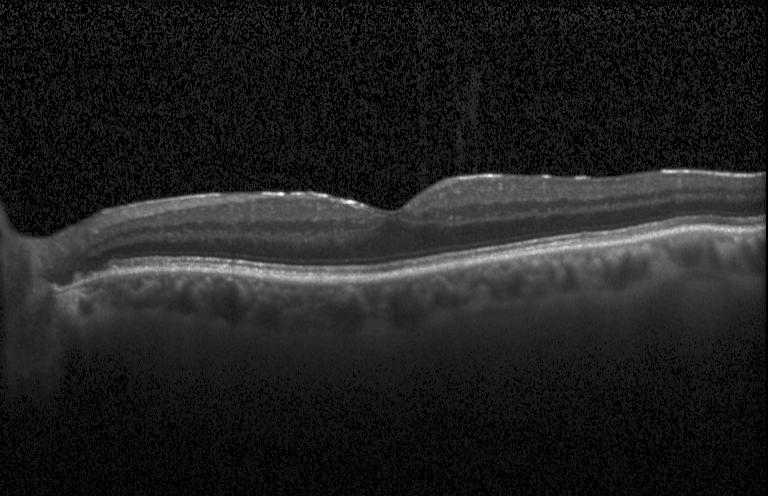 OCT line scan. Dx: no choroidal neovascularization, diabetic macular edema, or drusen.